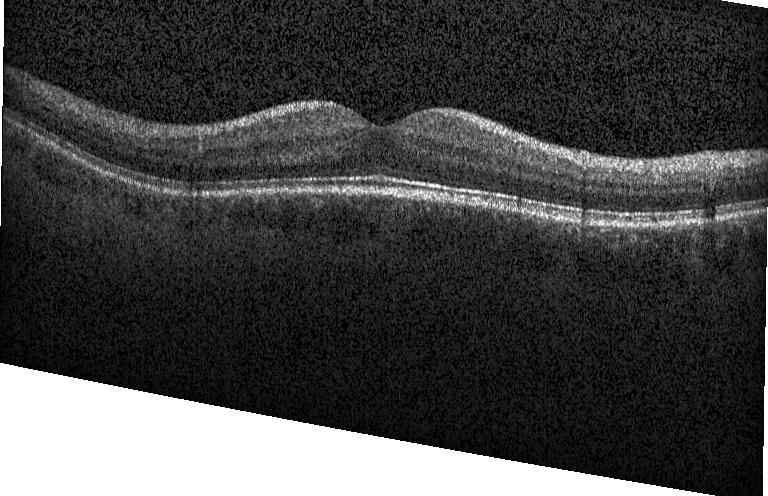

OCT B-scan.
OCT finding: neither CNV, DME, nor drusen.